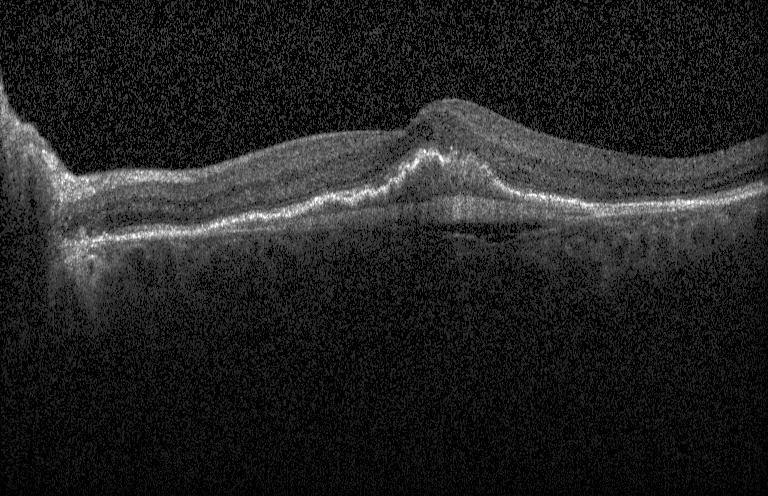
Retinal OCT B-scan, spectral-domain optical coherence tomography.
Macular OCT: CNV.